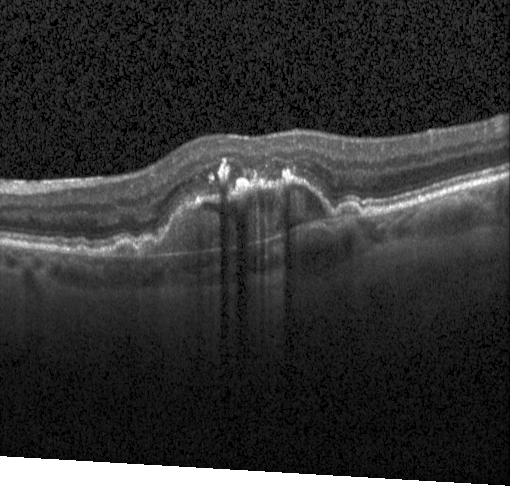
OCT B-scan. Instrument: Heidelberg Spectralis — Diagnosis: CNV.